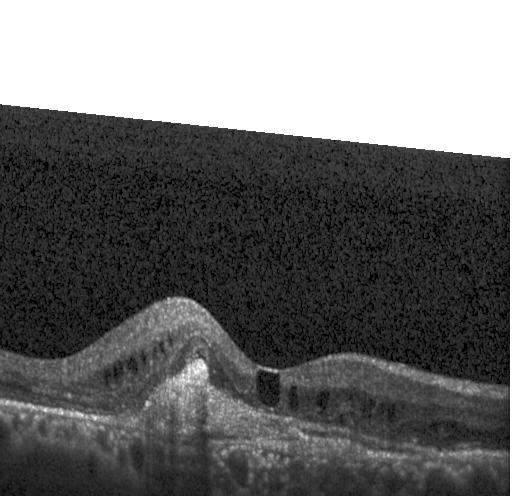
OCT line scan — Finding: choroidal neovascularization.